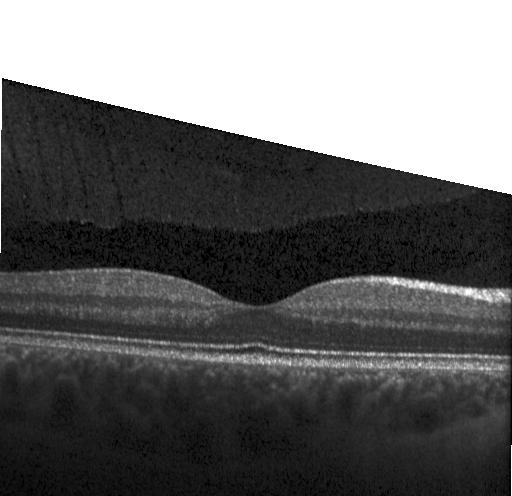

Optical coherence tomography scan. Diagnosis: neither choroidal neovascularization, diabetic macular edema, nor drusen.